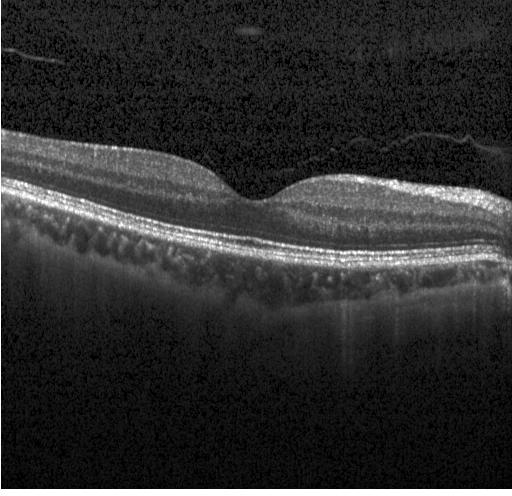
Centered on the fovea. Instrument: Heidelberg Spectralis. Retinal OCT B-scan. SD-OCT. Assessment: no CNV, DME, or drusen.